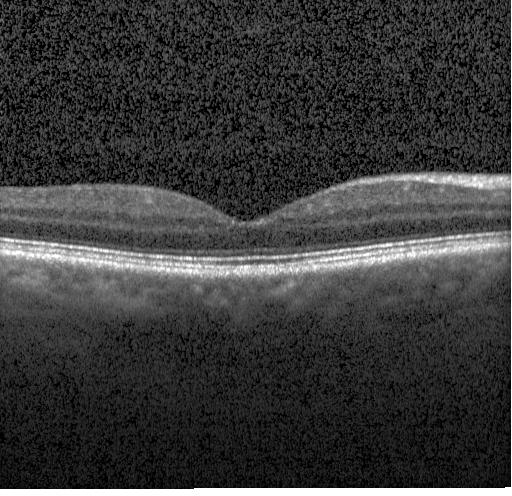 Spectral-domain OCT · OCT B-scan · macular scan · acquired on a Heidelberg Spectralis
This B-scan demonstrates no evidence of CNV, DME, or drusen.